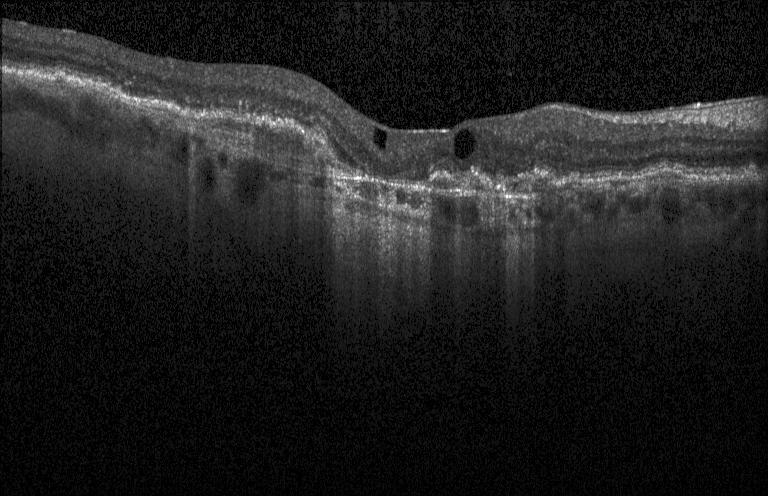
OCT B-scan; spectral-domain optical coherence tomography; acquired on a Heidelberg Spectralis. Diagnosis: a choroidal neovascular membrane.